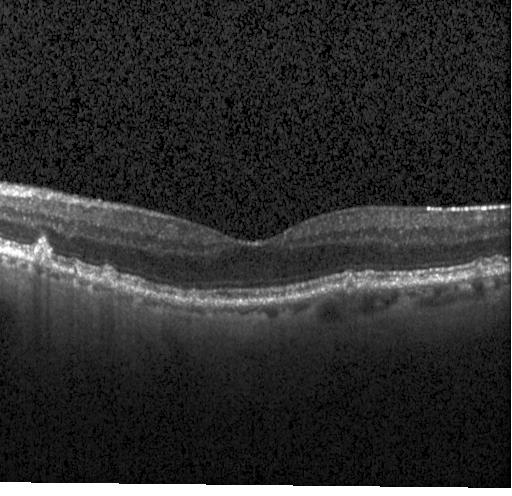
Multiple drusen.